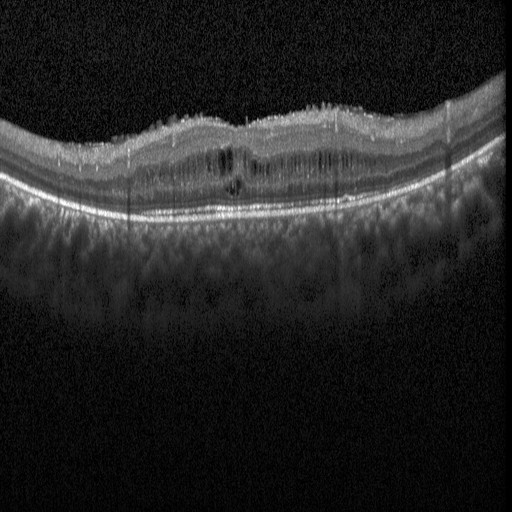
SD-OCT · OCT B-scan · Heidelberg Spectralis OCT system · through the macula. Impression: DME.